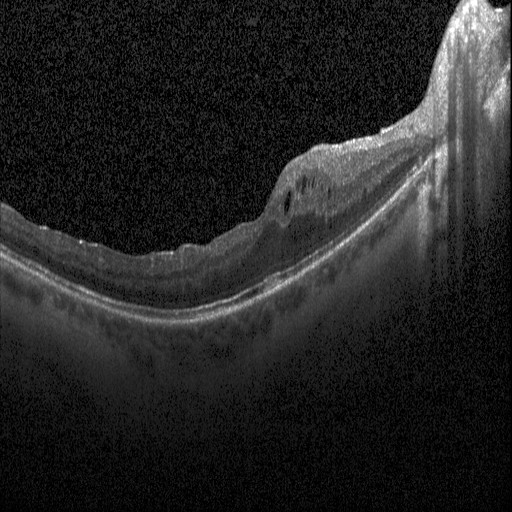

This B-scan demonstrates DME.